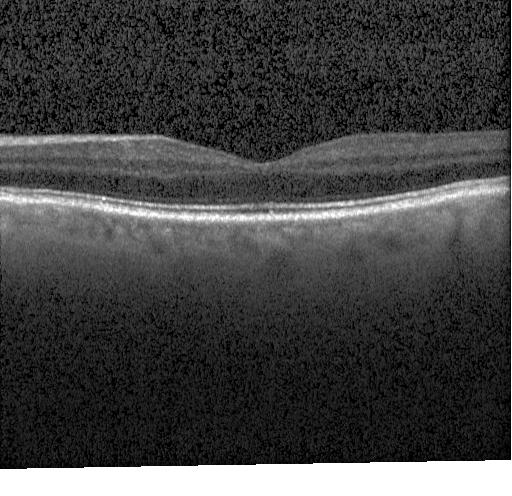

Finding: no choroidal neovascularization, diabetic macular edema, or drusen.